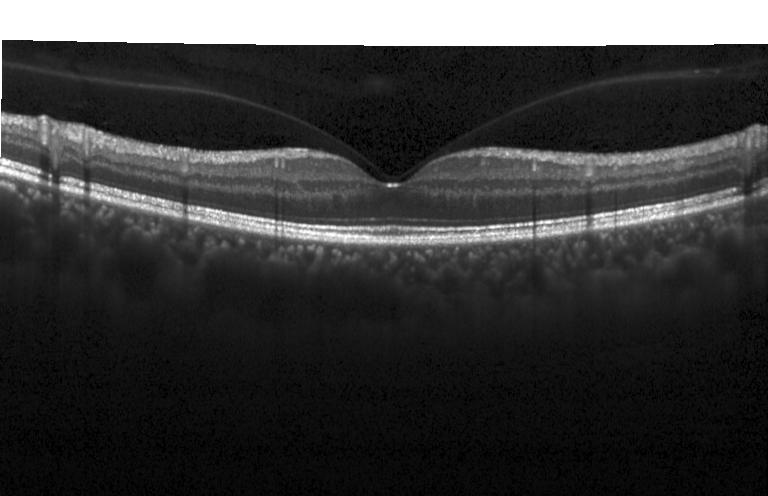
This B-scan demonstrates neither CNV, DME, nor drusen.